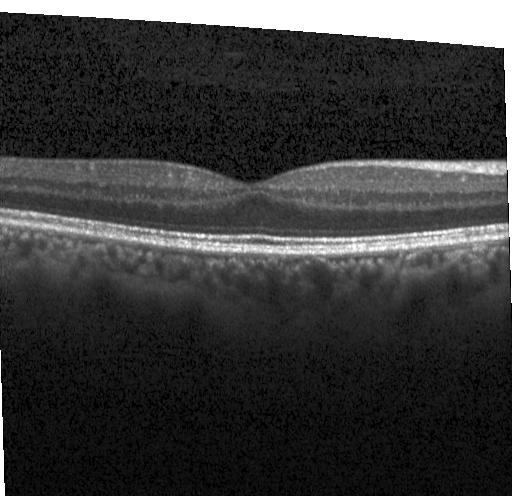

Acquired on a Heidelberg Spectralis · optical coherence tomography scan · fovea-centered · SD-OCT. Finding: no evidence of choroidal neovascularization, diabetic macular edema, or drusen.